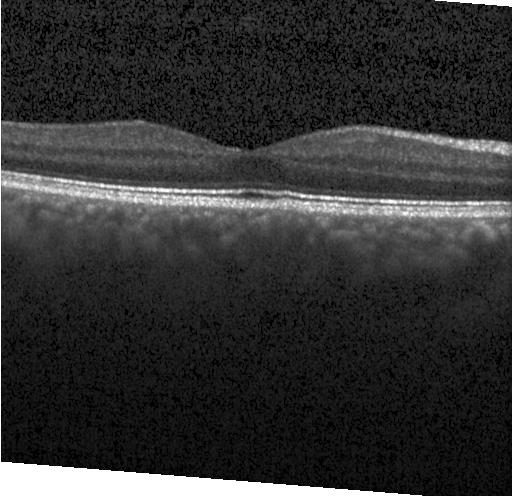
OCT line scan, macular scan.
Macular OCT: no evidence of choroidal neovascularization, diabetic macular edema, or drusen.